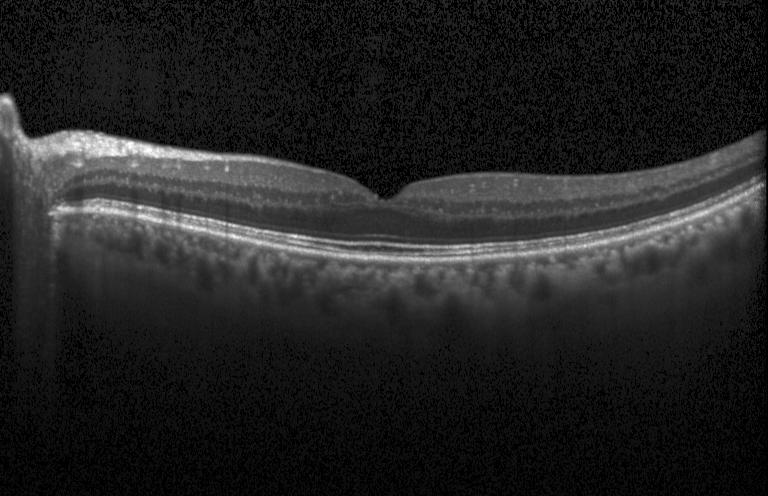

OCT line scan. Through the macula — Impression: no evidence of choroidal neovascularization, diabetic macular edema, or drusen.